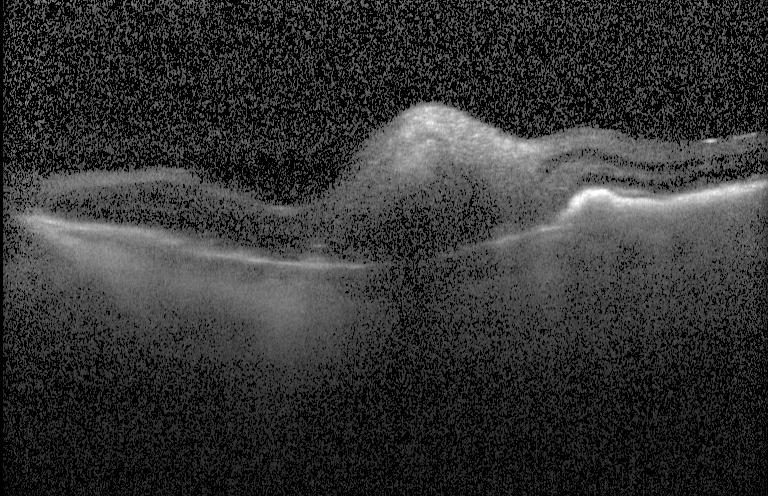
Diagnosis: CNV.